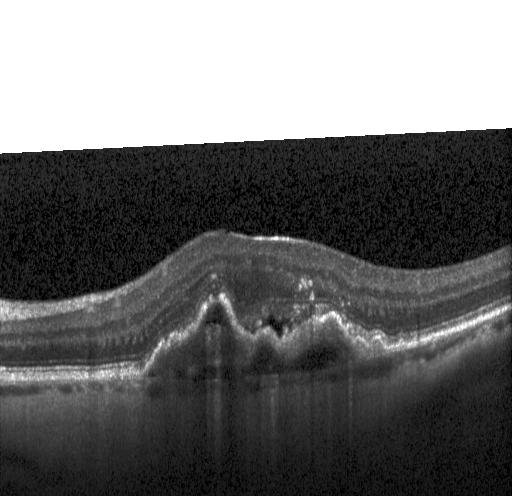
Retinal OCT B-scan. Acquired on a Heidelberg Spectralis
Finding: a choroidal neovascular membrane.